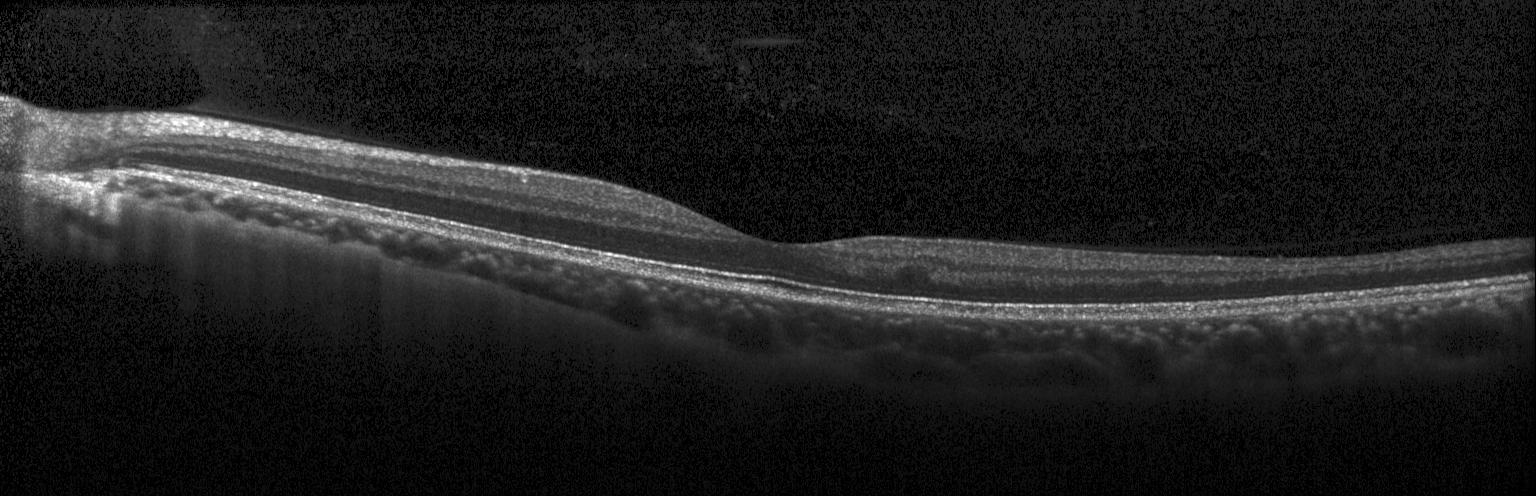 Impression: no choroidal neovascularization, diabetic macular edema, or drusen.